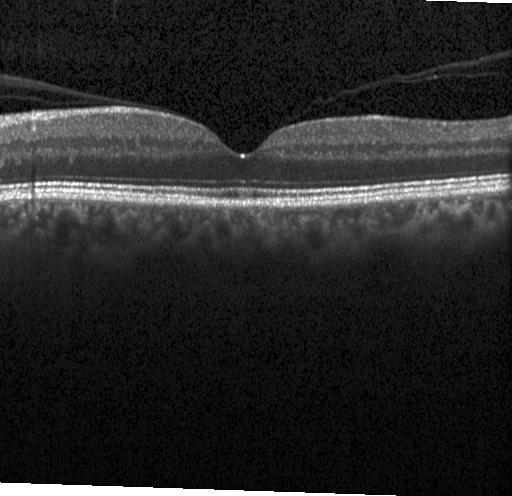

Optical coherence tomography B-scan · instrument: Heidelberg Spectralis · spectral-domain optical coherence tomography.
Finding: no choroidal neovascularization, no diabetic macular edema, and no drusen.